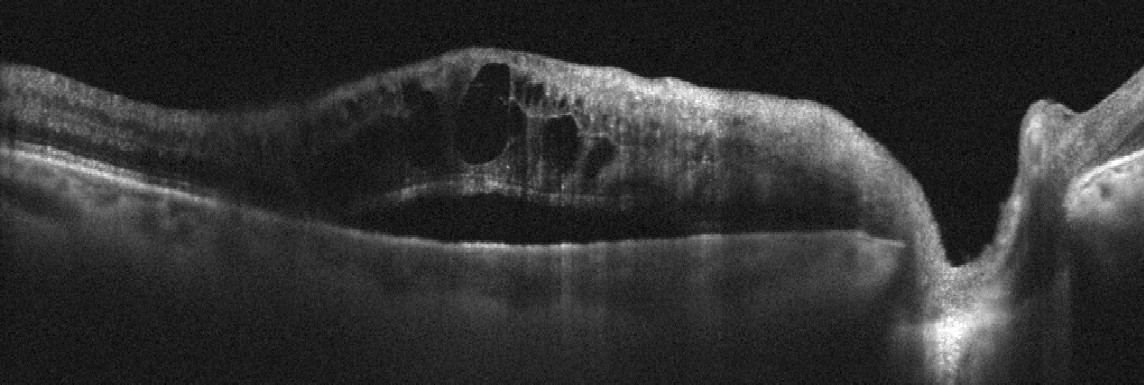

This B-scan demonstrates retinal vein occlusion (RVO).